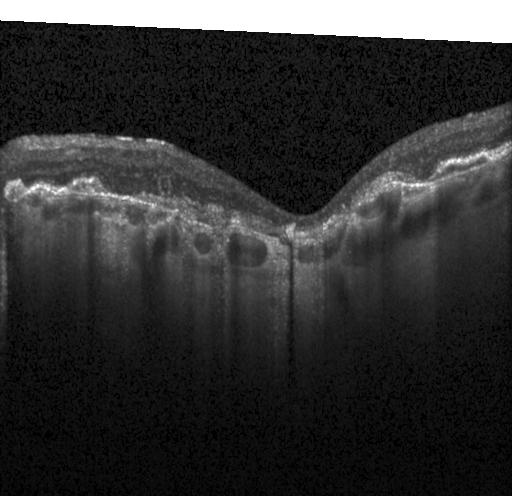

OCT scan showing a choroidal neovascular membrane.